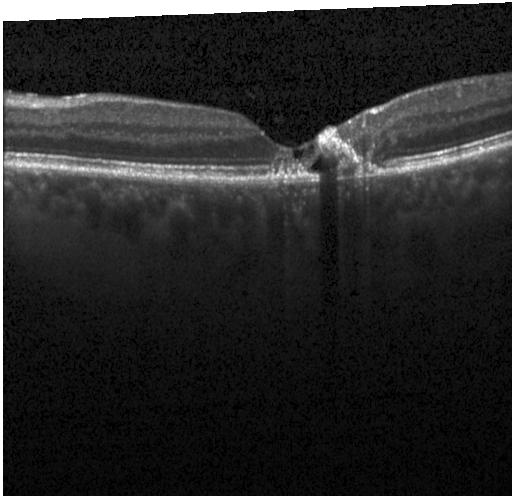

Diagnosis: a choroidal neovascular membrane.